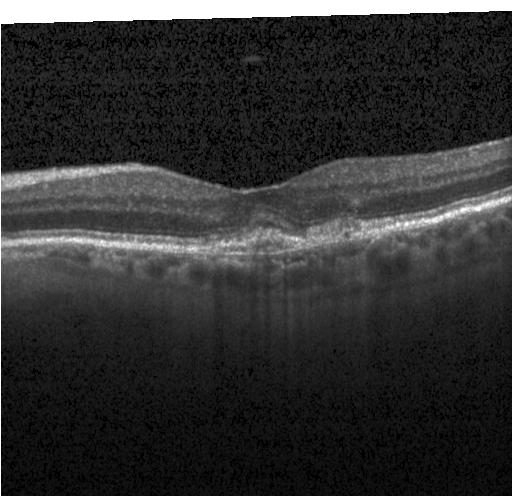

Spectral-domain OCT B-scan: a choroidal neovascular membrane.